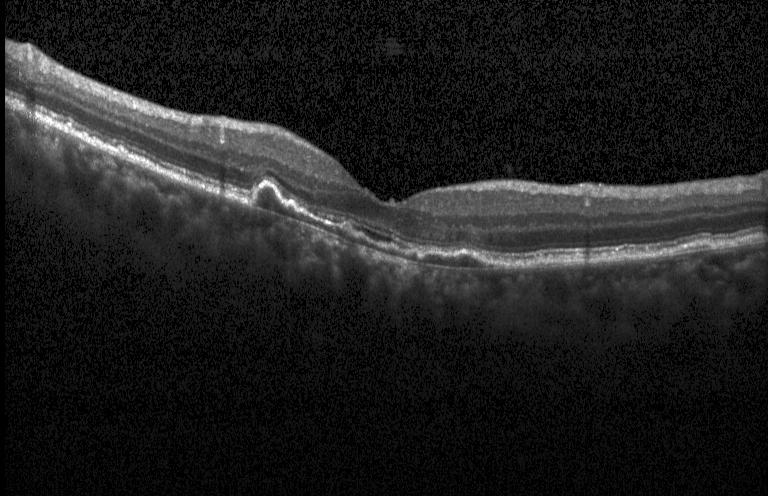
Optical coherence tomography B-scan. Heidelberg Spectralis OCT system. SD-OCT. Horizontal scan through the fovea.
Dx: a choroidal neovascular membrane.